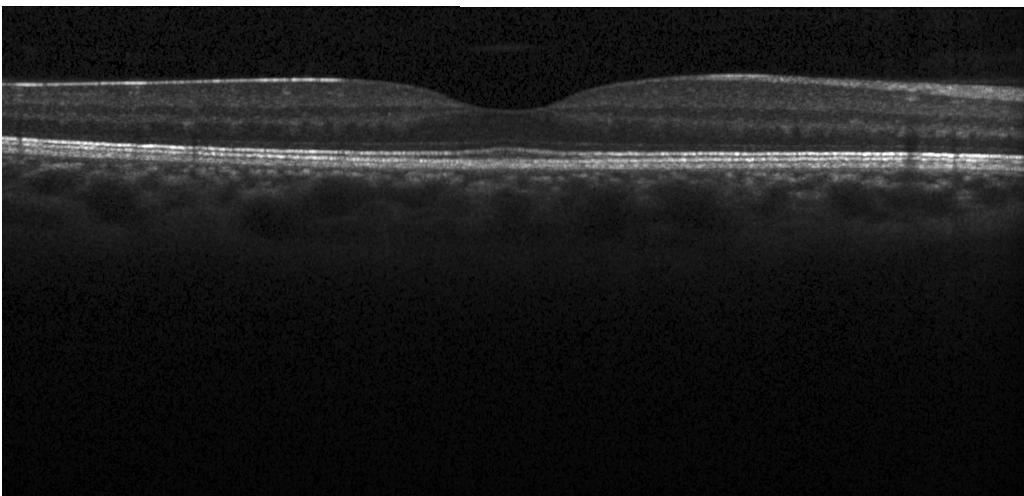 Diagnosis: no choroidal neovascularization, diabetic macular edema, or drusen.